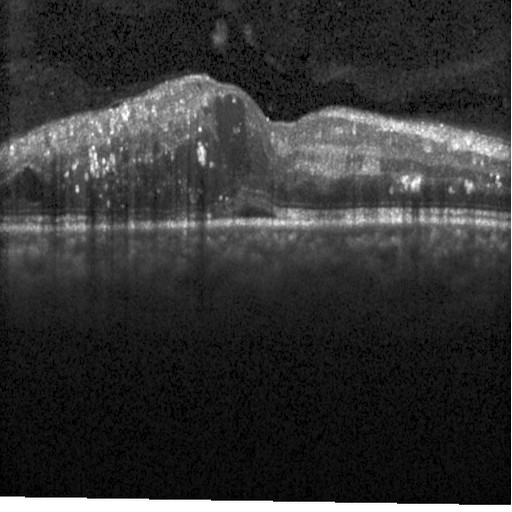

Retinal OCT cross-section showing diabetic macular edema.